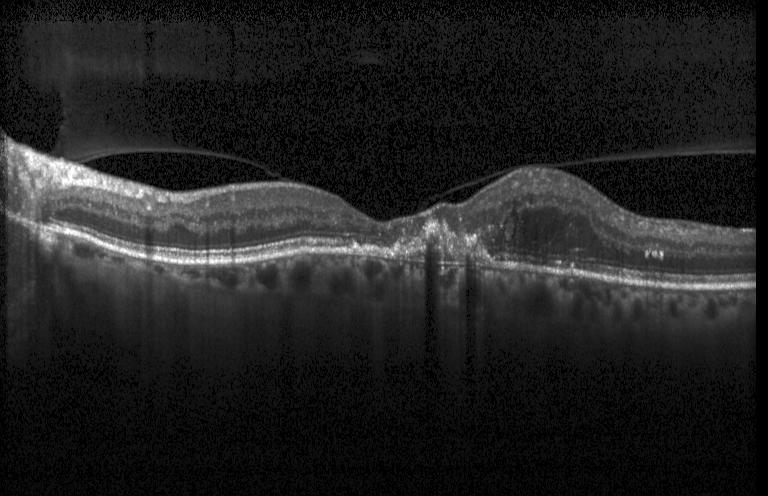 Assessment: CNV.